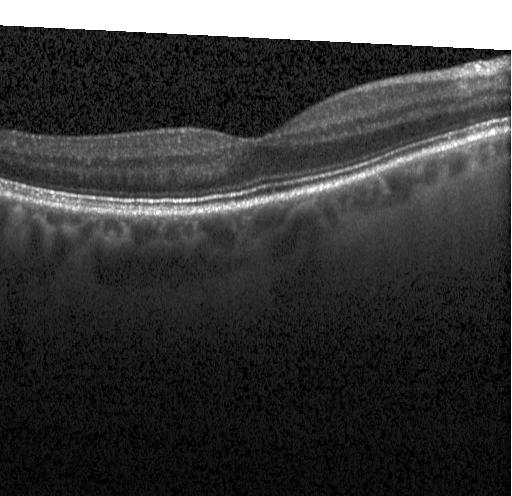

No CNV, no DME, and no drusen.